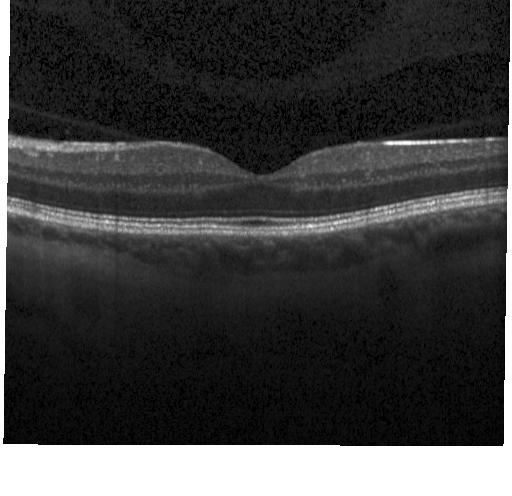
This B-scan demonstrates no evidence of choroidal neovascularization, diabetic macular edema, or drusen.